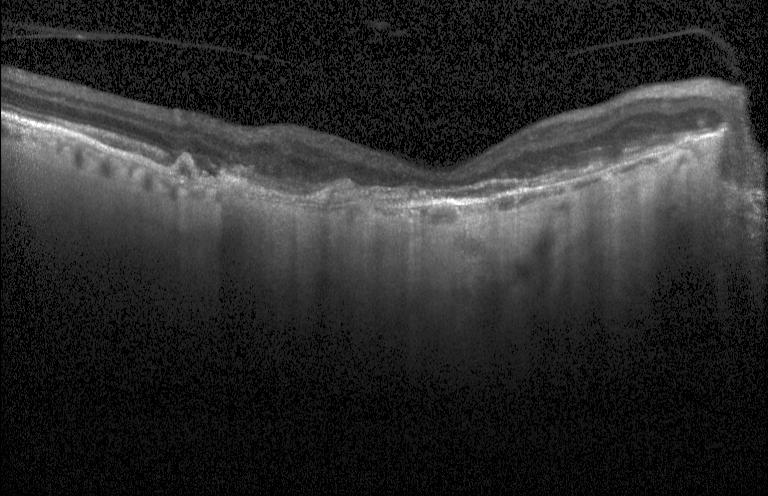 The scan shows a choroidal neovascular membrane.